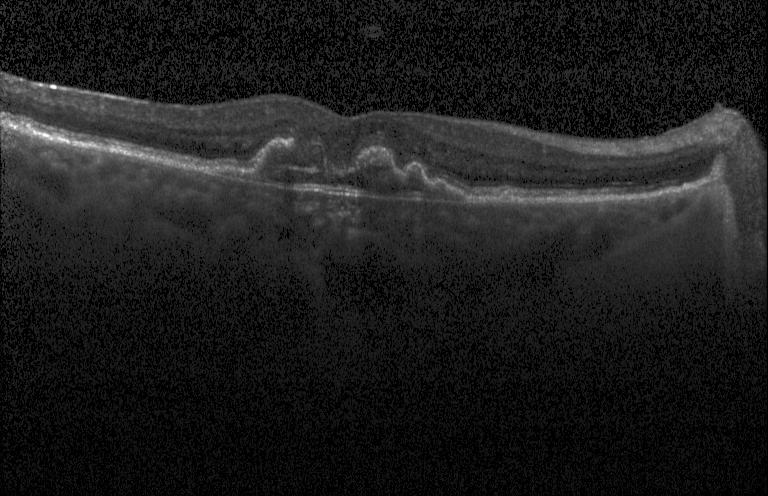
Impression: choroidal neovascularization (CNV).